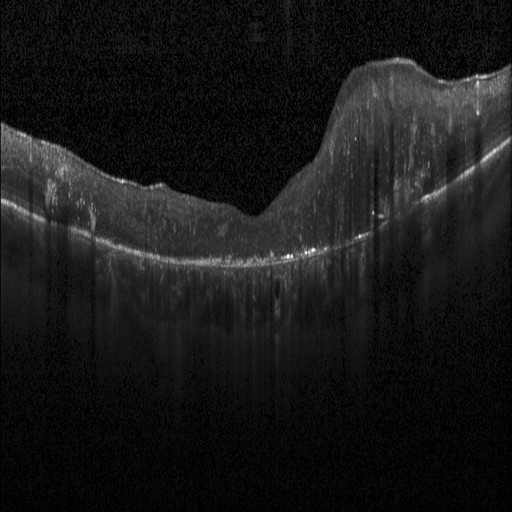 Diabetic macular edema (DME).